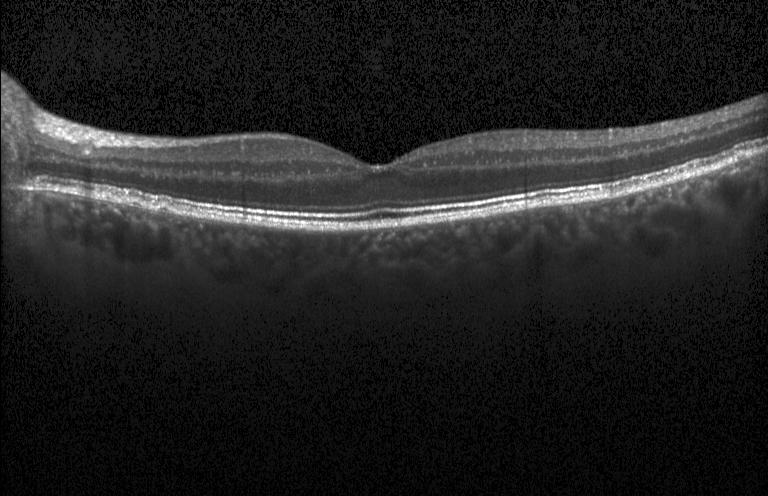 Spectral-domain optical coherence tomography · acquired on a Heidelberg Spectralis · centered on the fovea · retinal OCT B-scan
OCT finding: neither CNV, DME, nor drusen.